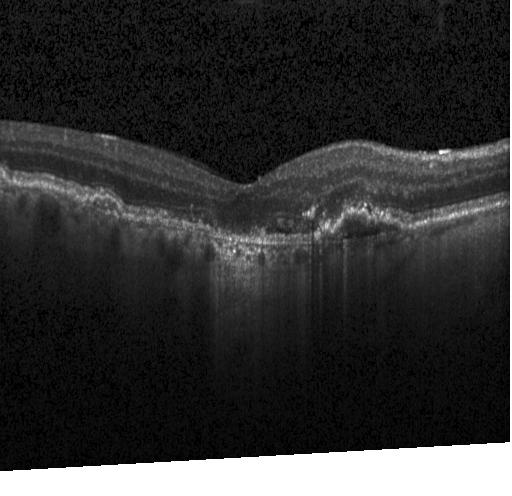
OCT scan showing choroidal neovascularization.